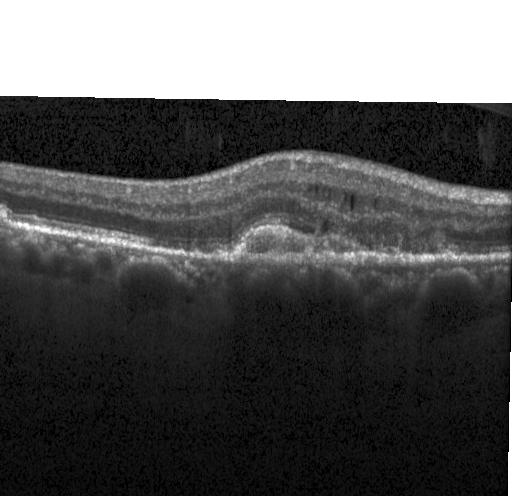
This B-scan demonstrates a choroidal neovascular membrane.